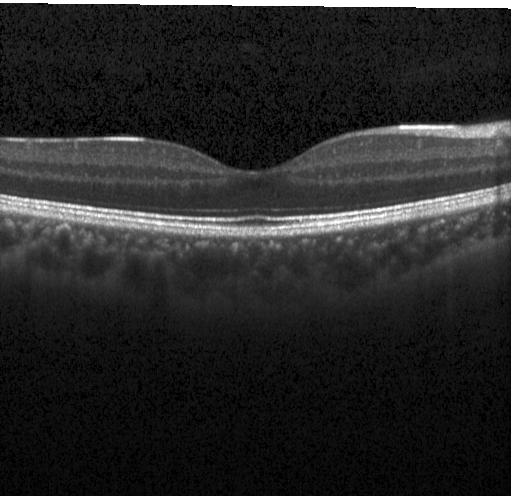

Optical coherence tomography scan, SD-OCT — No evidence of choroidal neovascularization, diabetic macular edema, or drusen.